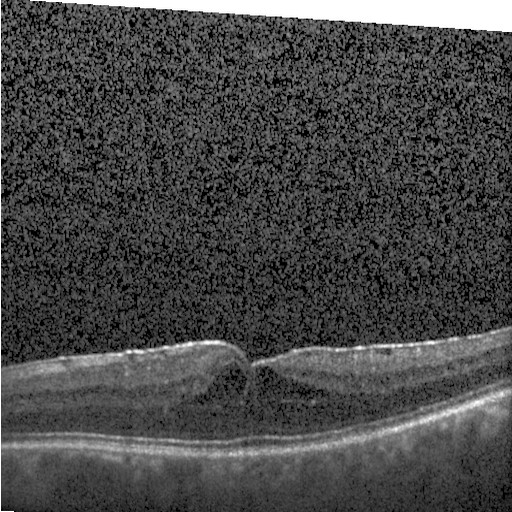
Spectral-domain OCT; optical coherence tomography scan — Impression: DME.